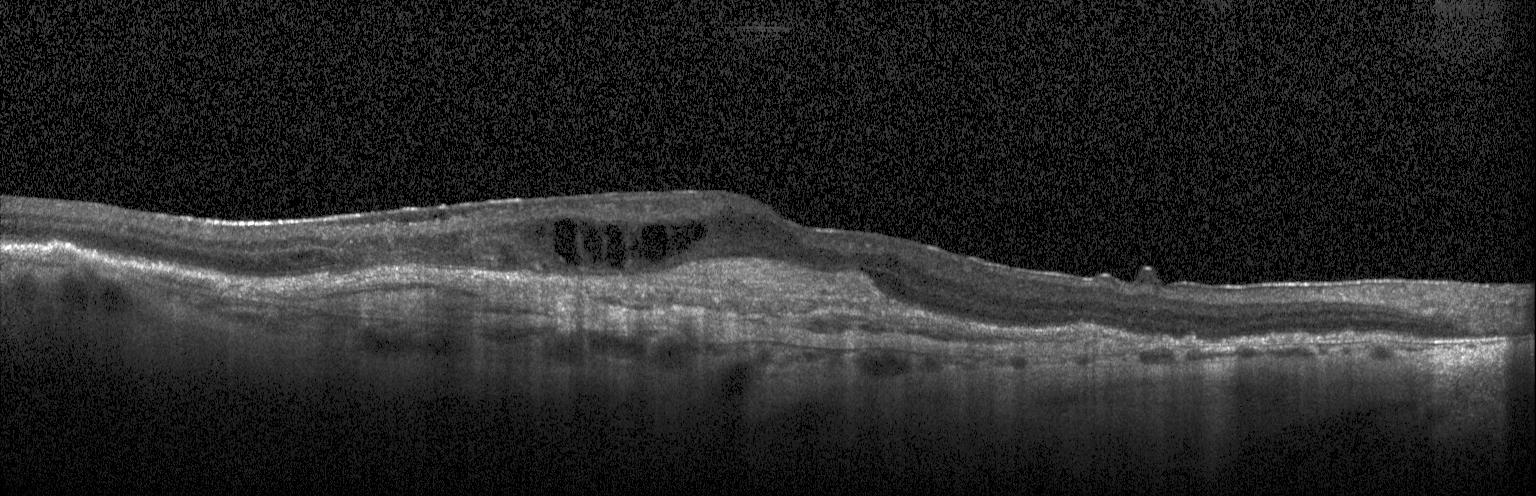 Retinal OCT B-scan.
Diagnosis: choroidal neovascularization (CNV).